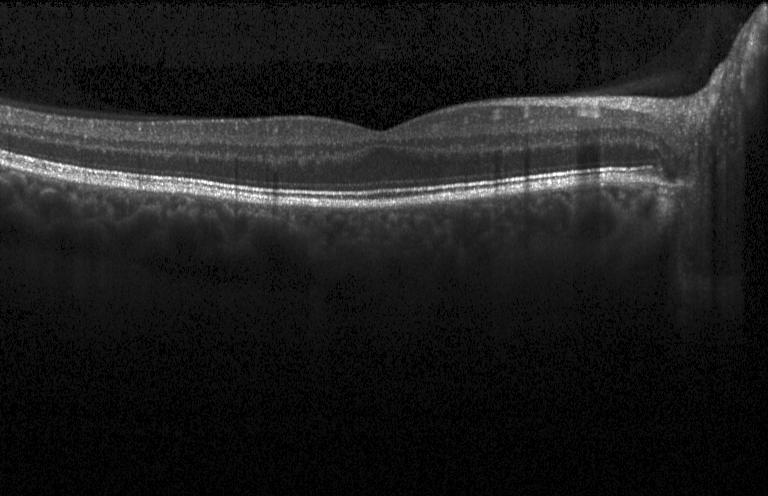 Heidelberg Spectralis; optical coherence tomography B-scan; macular scan — Impression: neither choroidal neovascularization, diabetic macular edema, nor drusen.